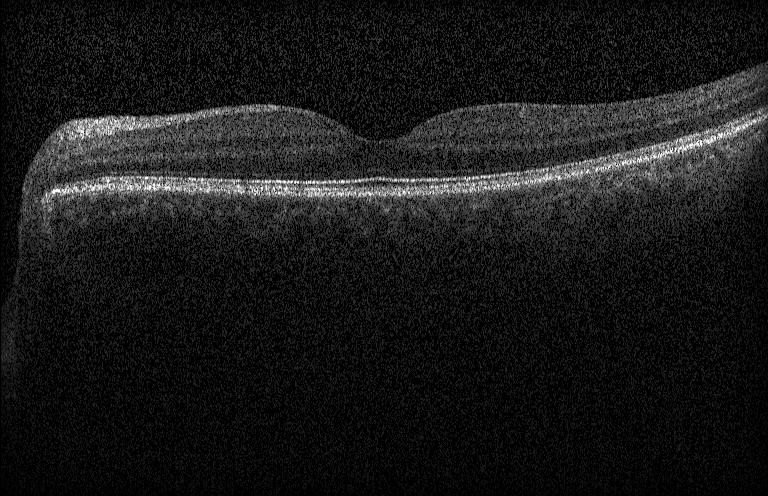
Horizontal scan through the fovea · spectral-domain OCT · OCT line scan. Impression: no CNV, DME, or drusen.